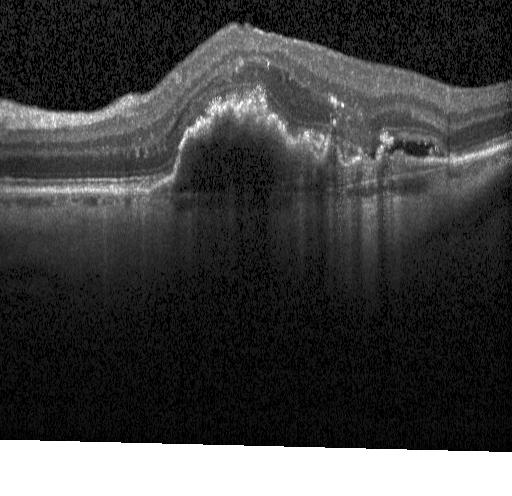

Spectral-domain OCT, OCT line scan, Heidelberg Spectralis, centered on the fovea — Diagnosis: choroidal neovascularization (CNV).